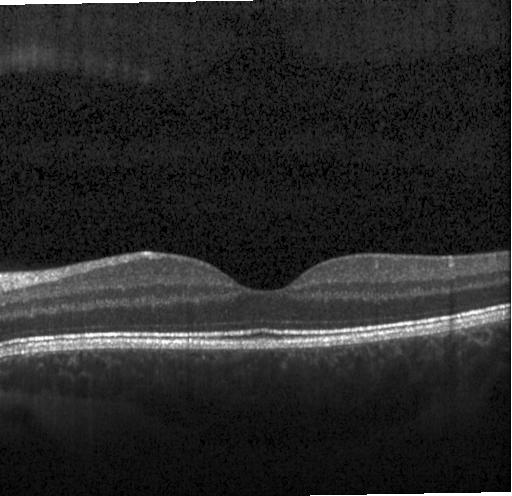 SD-OCT. Retinal OCT cross-section
Finding: no choroidal neovascularization, diabetic macular edema, or drusen.